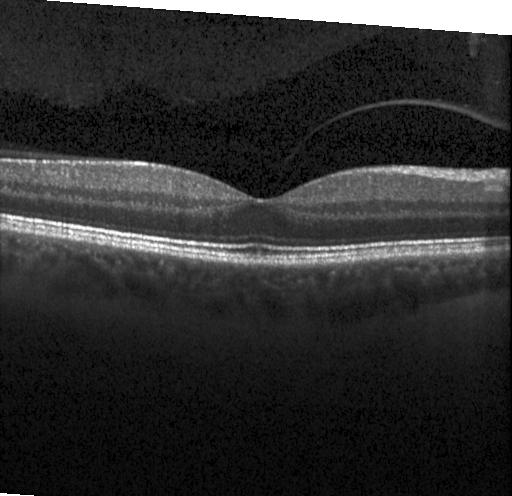 Diagnosis: no choroidal neovascularization, diabetic macular edema, or drusen.